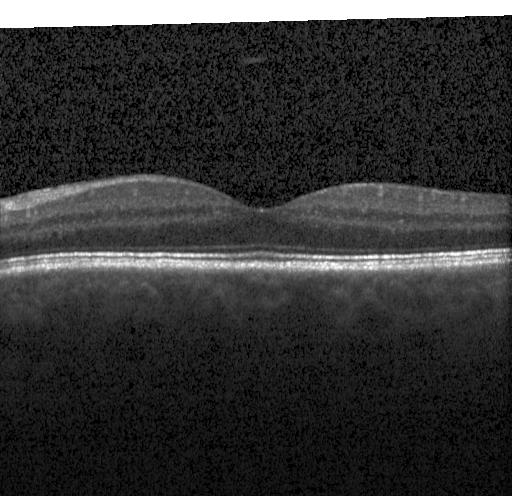 Impression: neither choroidal neovascularization, diabetic macular edema, nor drusen.